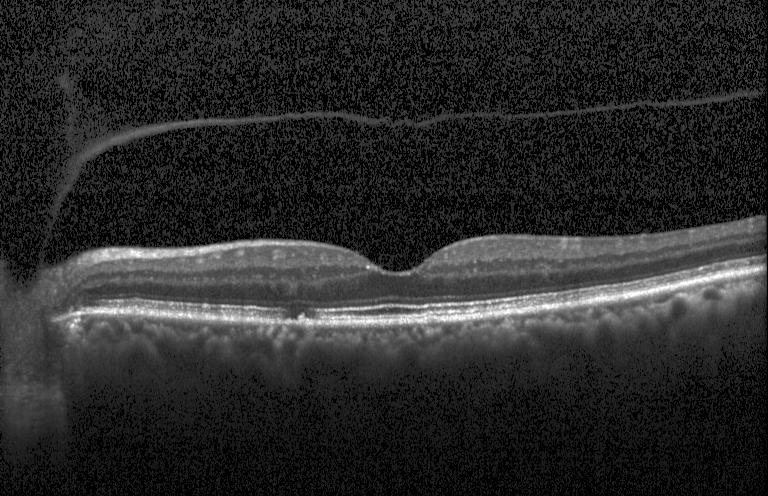

Optical coherence tomography B-scan, macular scan, SD-OCT, instrument: Heidelberg Spectralis — Assessment: sub-RPE drusenoid deposits.